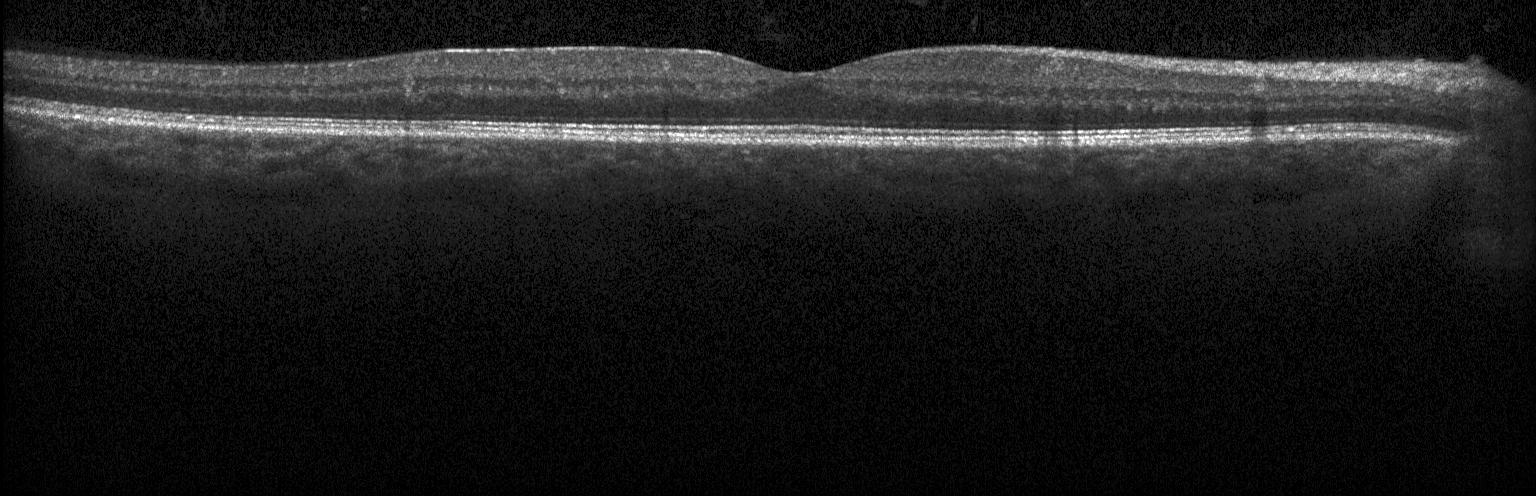

Finding: no evidence of choroidal neovascularization, diabetic macular edema, or drusen.